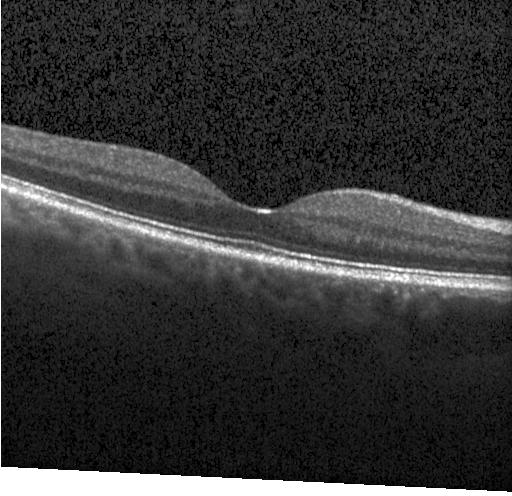
Retinal OCT B-scan — Diagnosis: no choroidal neovascularization, no diabetic macular edema, and no drusen.